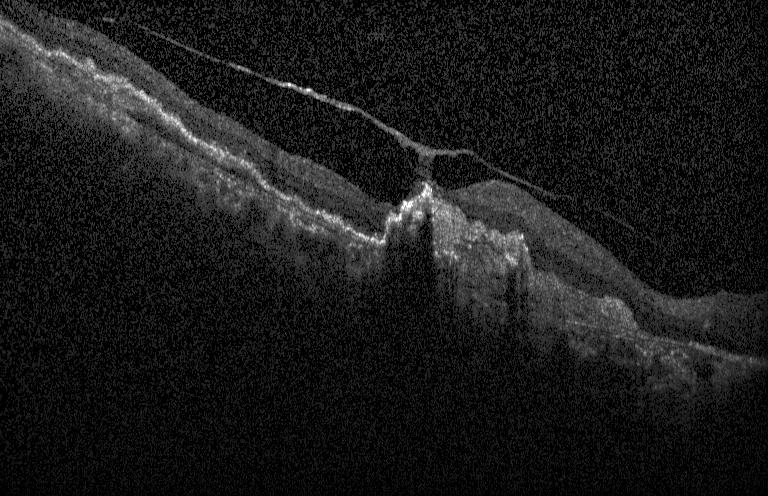

Retinal OCT B-scan — Choroidal neovascularization.